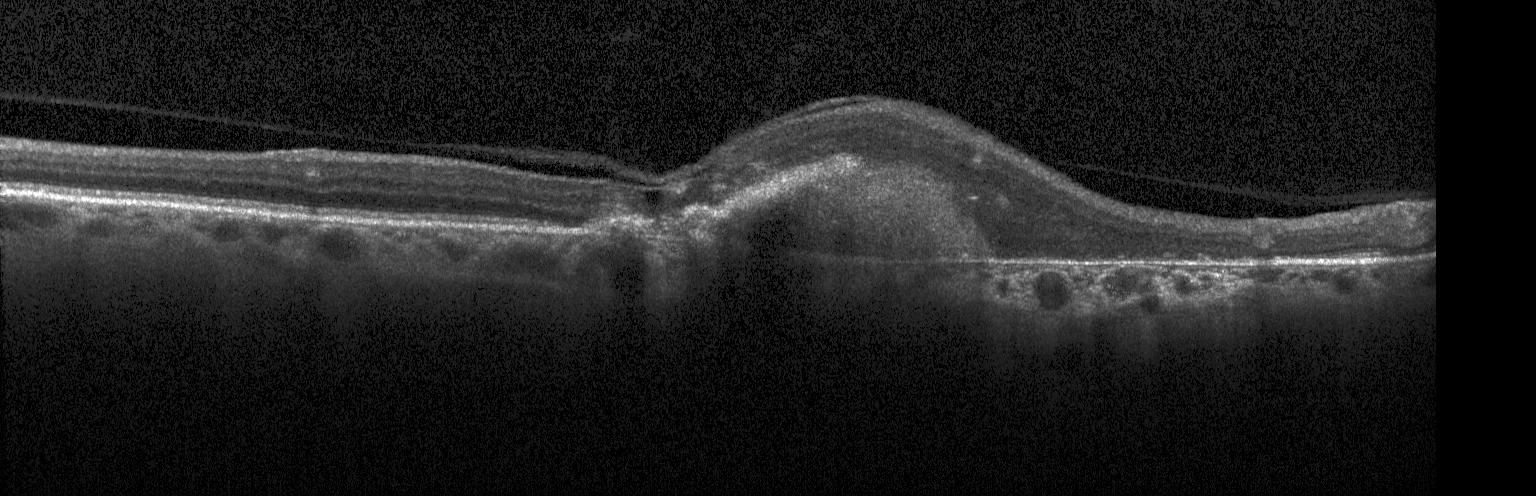 Impression: a choroidal neovascular membrane.